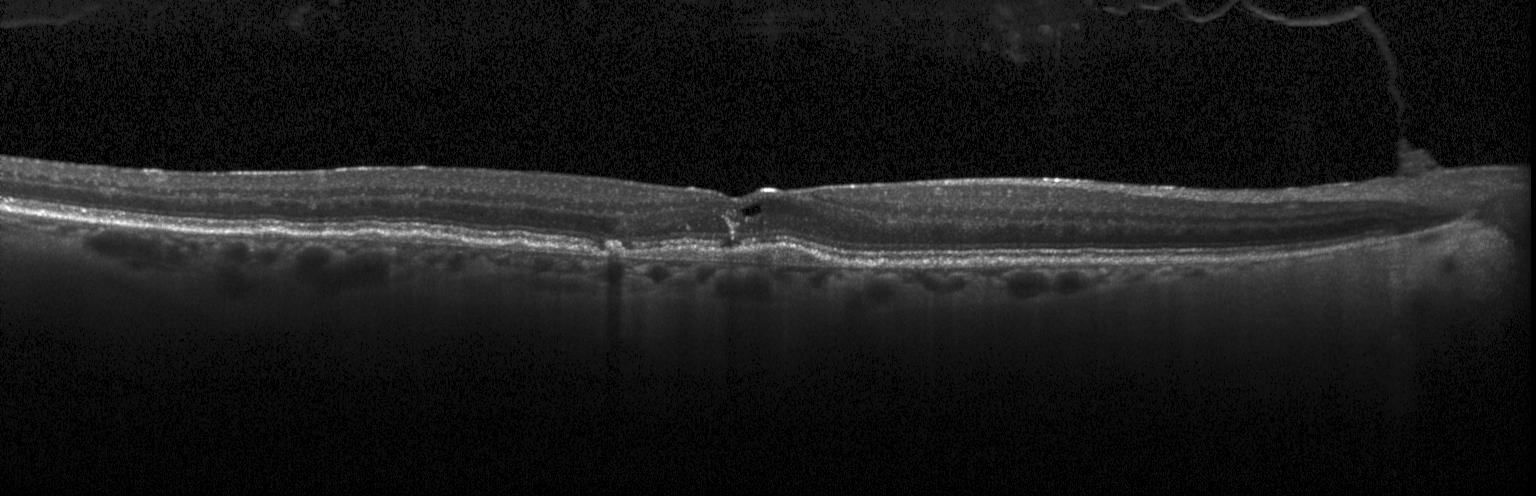

Impression: a choroidal neovascular membrane.